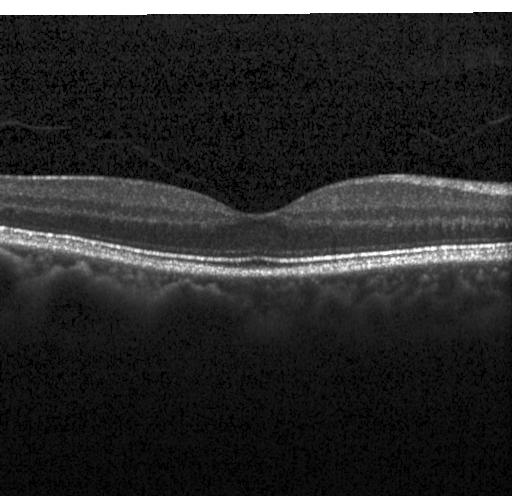
Finding: no CNV, no DME, and no drusen.